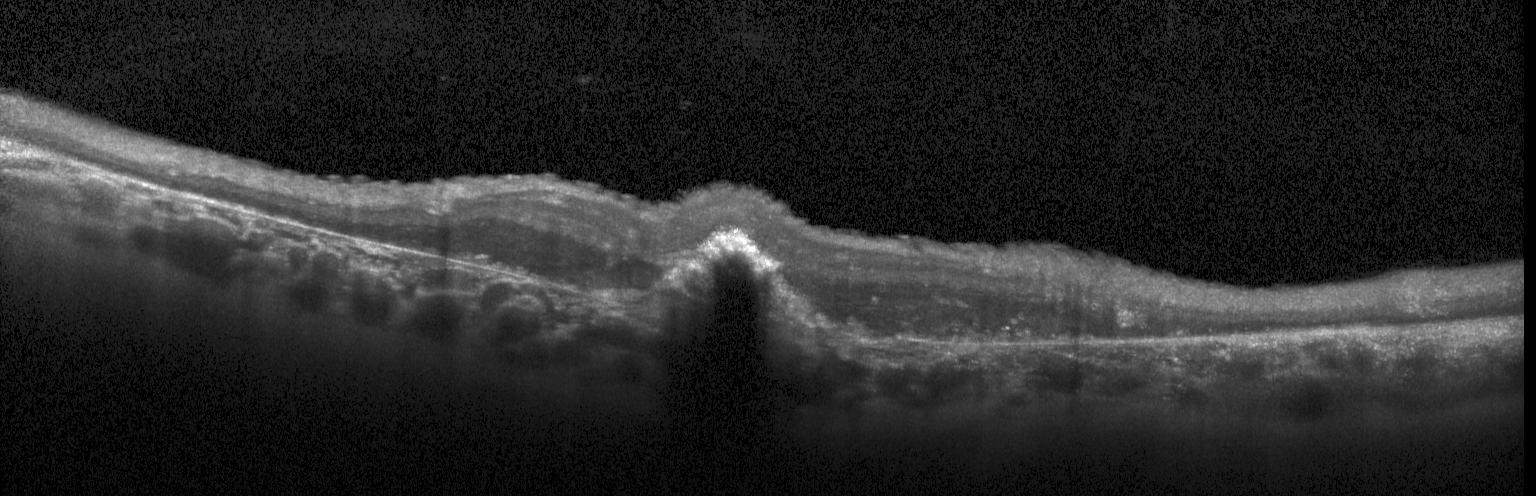 OCT scan showing choroidal neovascularization (CNV).